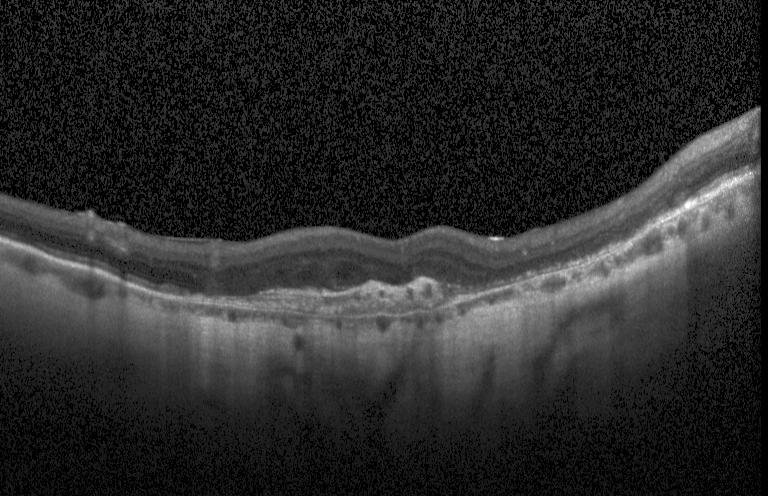 Finding: choroidal neovascularization.